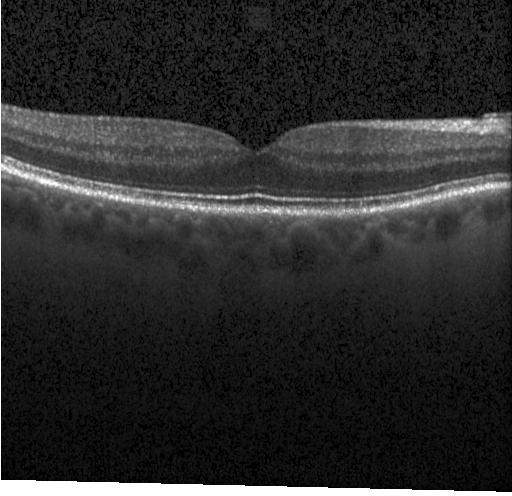

OCT B-scan showing no evidence of CNV, DME, or drusen.